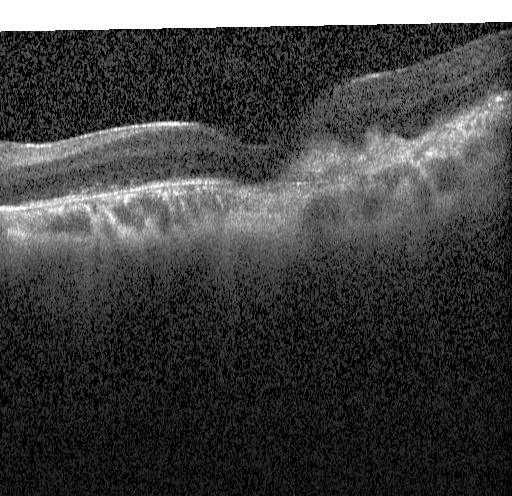

This B-scan demonstrates choroidal neovascularization.